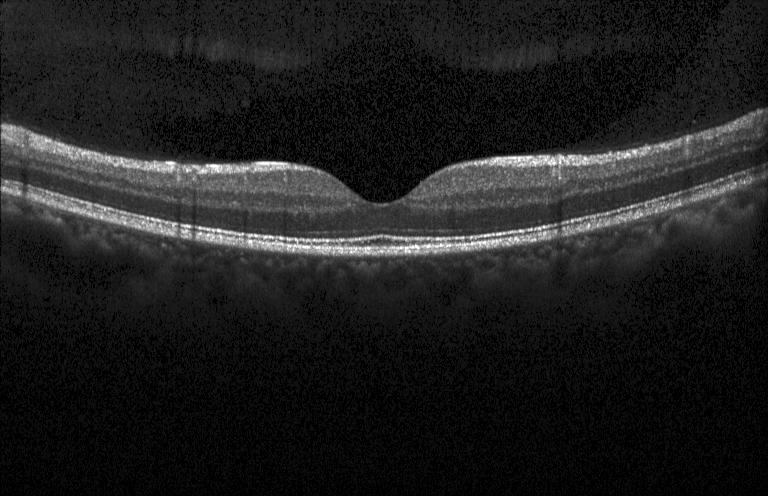 The scan shows no evidence of choroidal neovascularization, diabetic macular edema, or drusen.